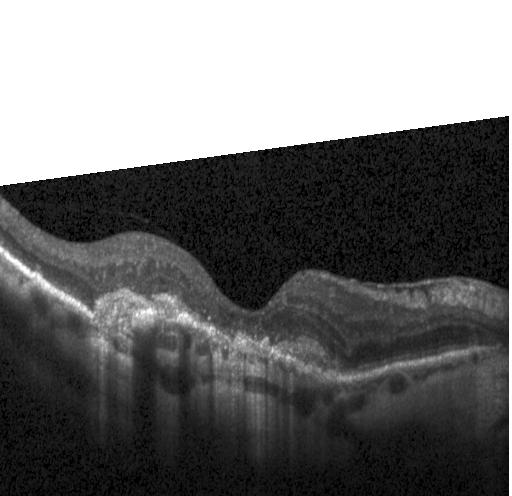

Heidelberg Spectralis OCT system · fovea-centered · OCT B-scan · SD-OCT — The scan shows CNV.